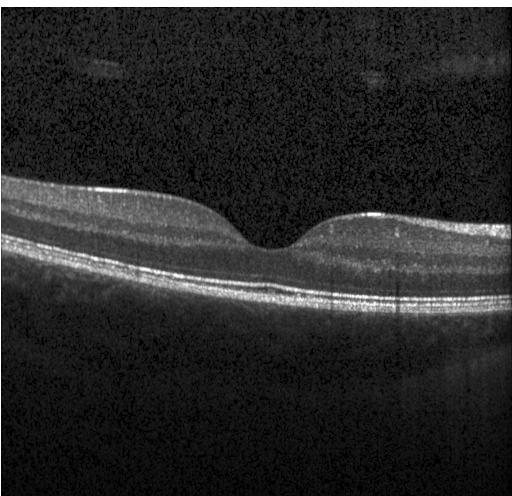
Impression: no evidence of choroidal neovascularization, diabetic macular edema, or drusen.